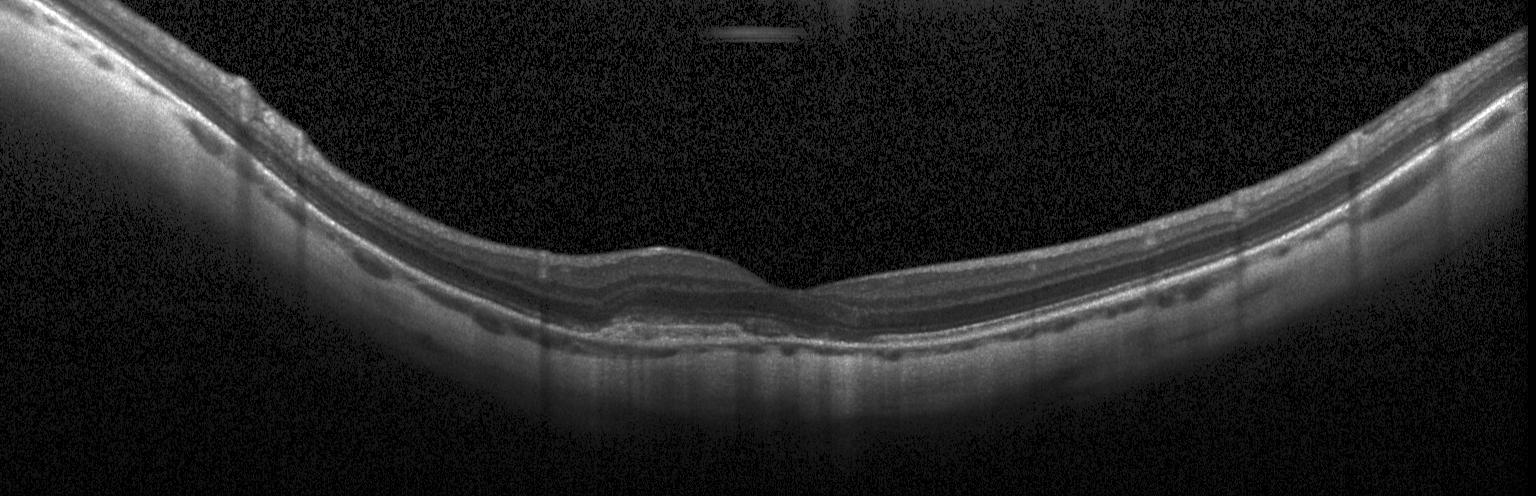
Acquired on a Heidelberg Spectralis. SD-OCT. Optical coherence tomography B-scan. Centered on the fovea — Impression: CNV.